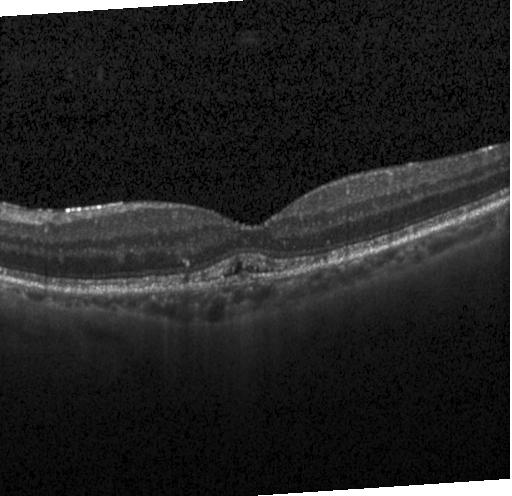
Acquired on a Heidelberg Spectralis. Centered on the fovea. Optical coherence tomography B-scan. Spectral-domain optical coherence tomography
Finding: a choroidal neovascular membrane.